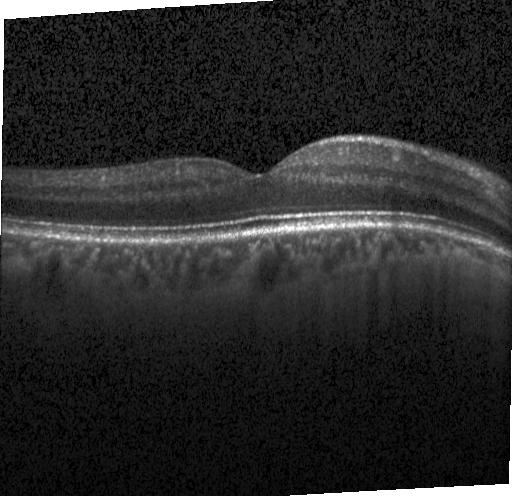
SD-OCT; retinal OCT B-scan; Heidelberg Spectralis; fovea-centered
The scan shows neither CNV, DME, nor drusen.